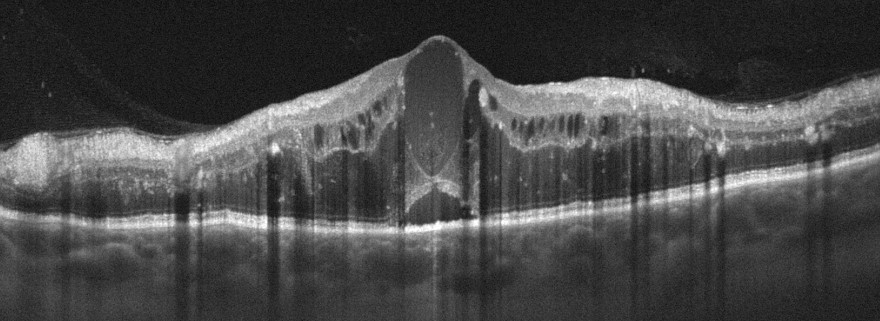

Optical coherence tomography B-scan
Dx: DME.